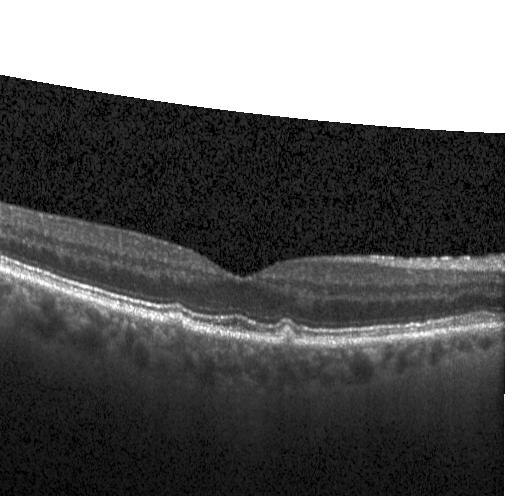
Horizontal scan through the fovea; acquired on a Heidelberg Spectralis; OCT B-scan
This B-scan demonstrates sub-RPE drusenoid deposits.